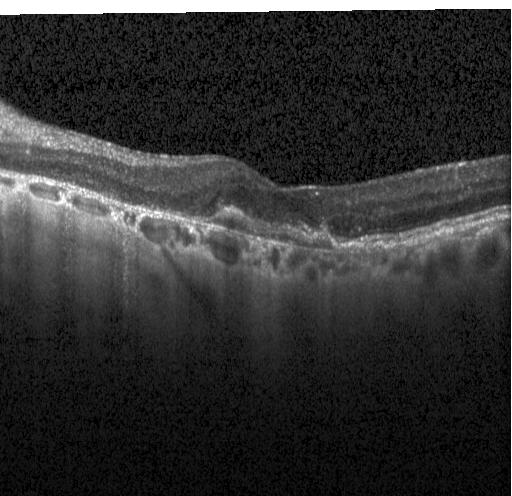 Horizontal scan through the fovea. Retinal OCT cross-section. SD-OCT
Assessment: choroidal neovascularization.